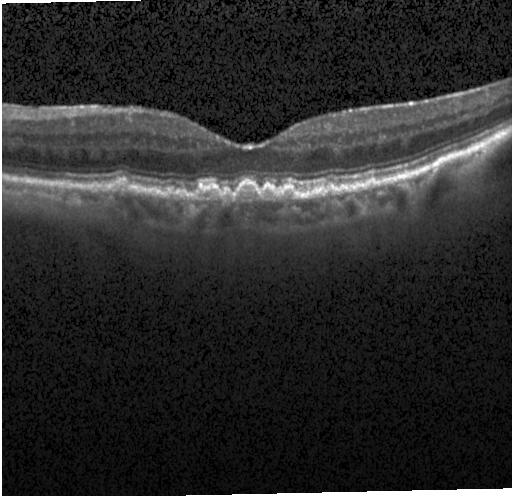 Retinal OCT cross-section
This B-scan demonstrates multiple drusen.